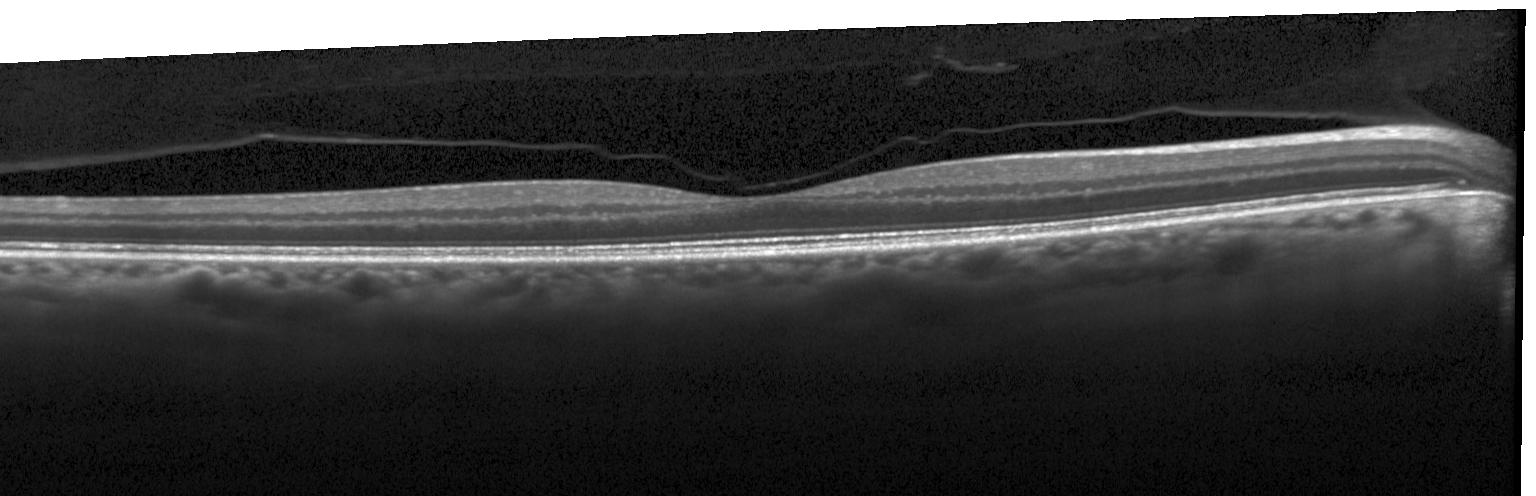
Spectral-domain optical coherence tomography. Macular scan. Heidelberg Spectralis. Optical coherence tomography scan
This B-scan demonstrates neither CNV, DME, nor drusen.